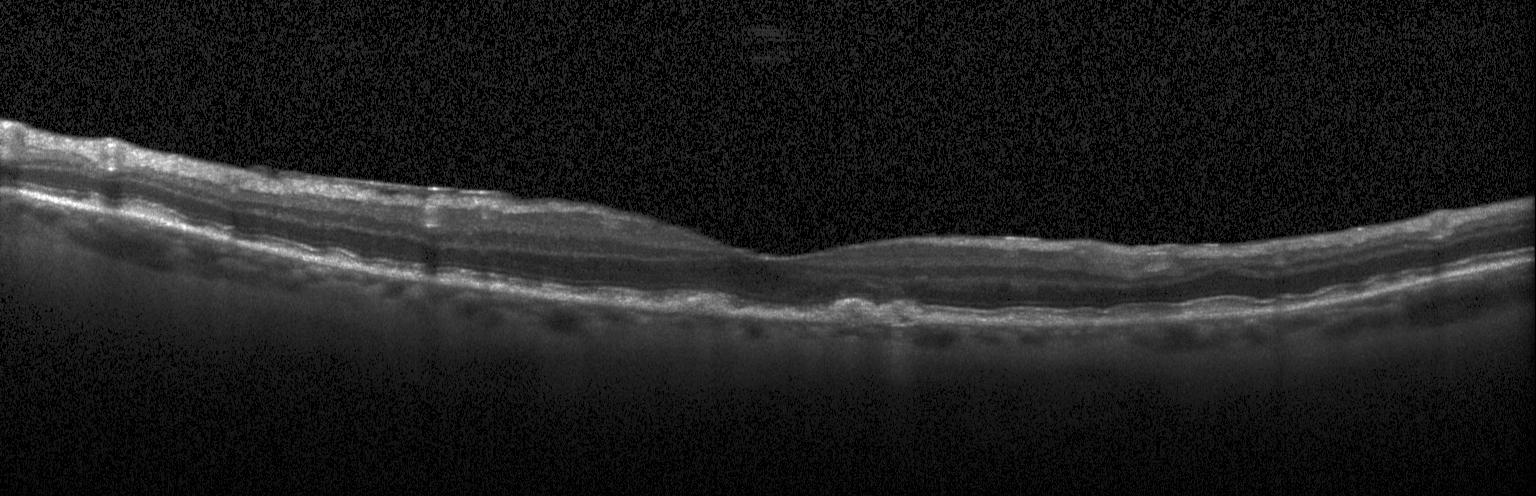

Diagnosis: drusen.